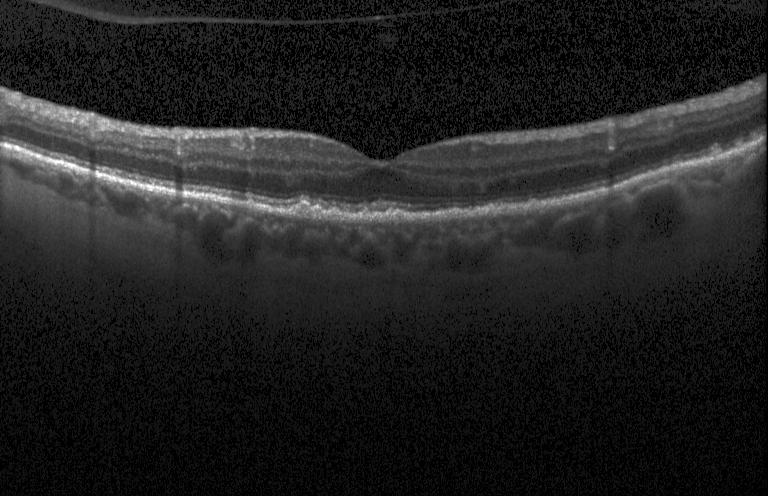 Macular OCT demonstrating sub-RPE drusenoid deposits.